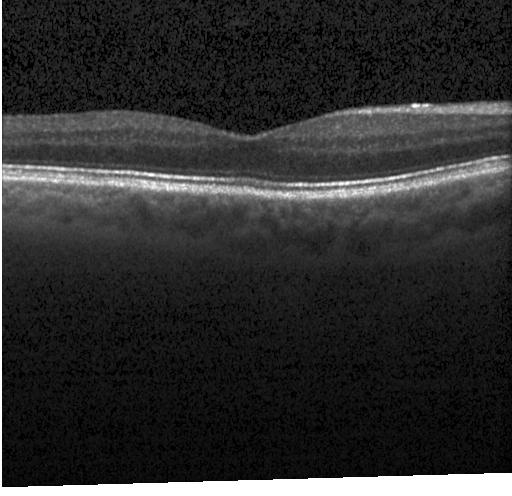

Heidelberg Spectralis. OCT B-scan. Macular scan. Spectral-domain optical coherence tomography.
The scan shows neither choroidal neovascularization, diabetic macular edema, nor drusen.